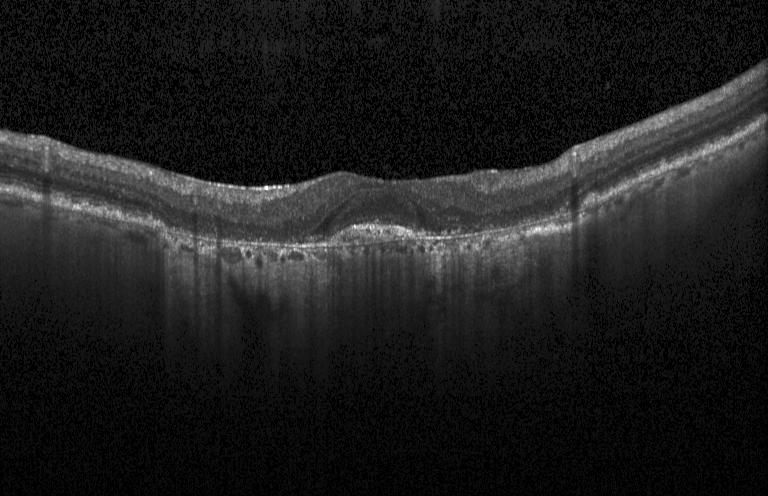

OCT B-scan showing a choroidal neovascular membrane.